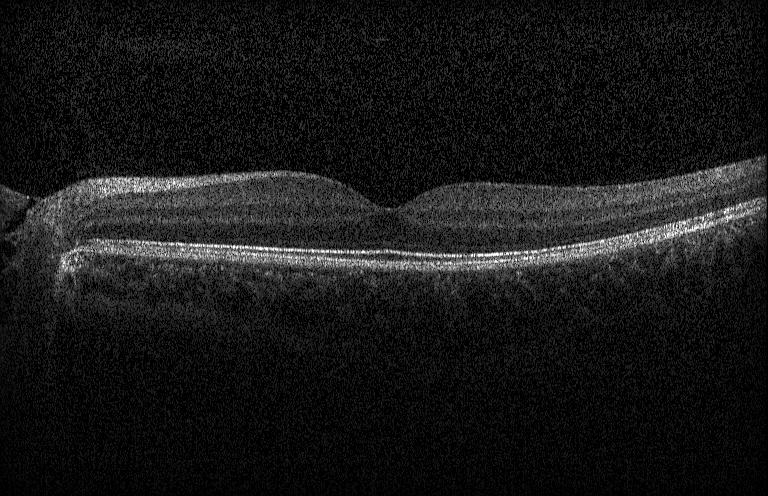
Finding: neither choroidal neovascularization, diabetic macular edema, nor drusen.